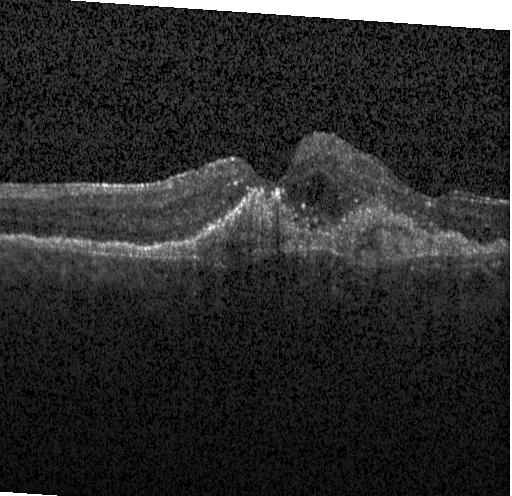

Dx: choroidal neovascularization.